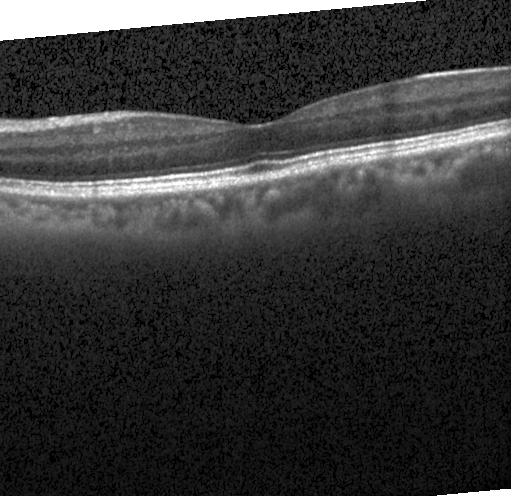
Optical coherence tomography scan. Heidelberg Spectralis OCT system — Diagnosis: no CNV, no DME, and no drusen.